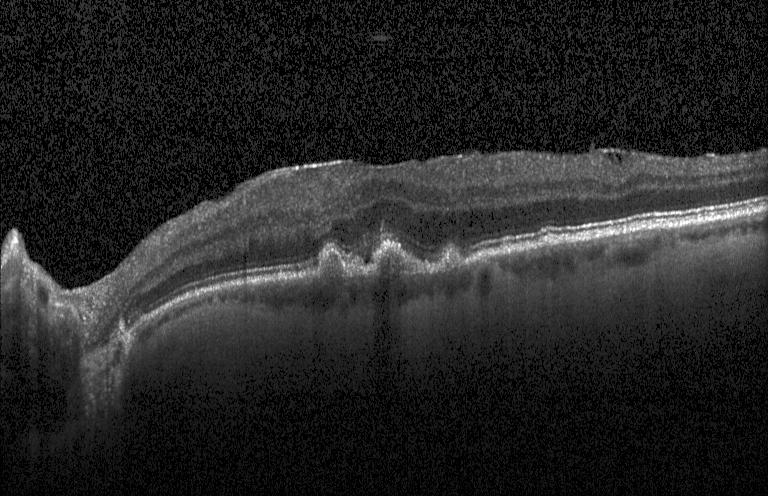
OCT B-scan showing sub-RPE drusenoid deposits.